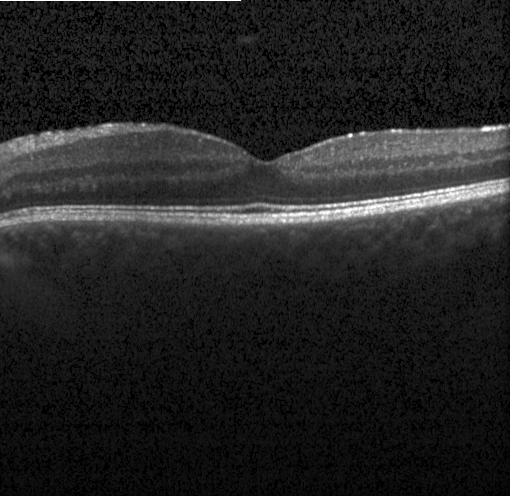 Spectral-domain OCT B-scan: no choroidal neovascularization, no diabetic macular edema, and no drusen.